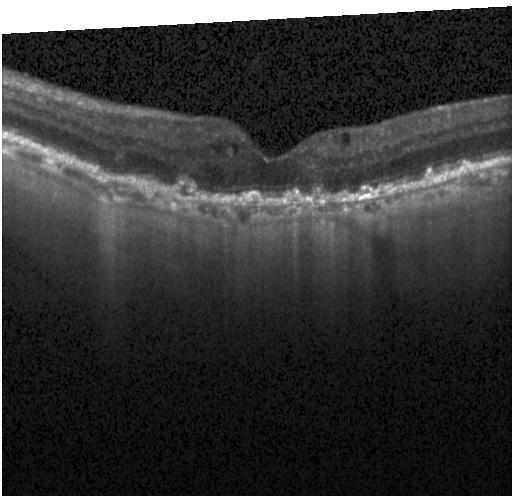
This B-scan demonstrates choroidal neovascularization (CNV).